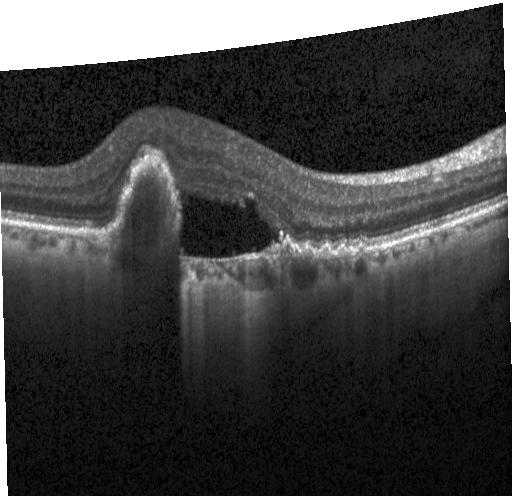

Spectral-domain optical coherence tomography · retinal OCT cross-section · macular scan. Impression: a choroidal neovascular membrane.